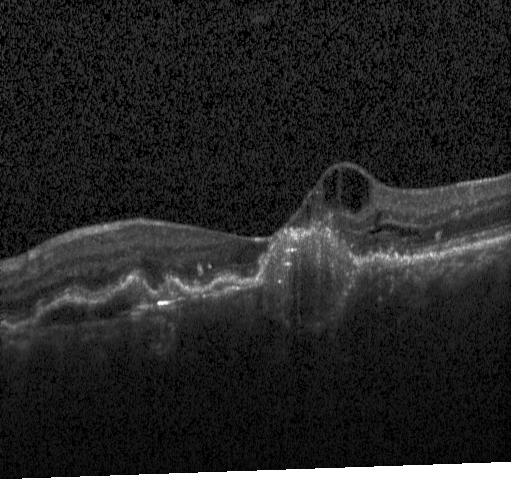 Macular OCT demonstrating a choroidal neovascular membrane.